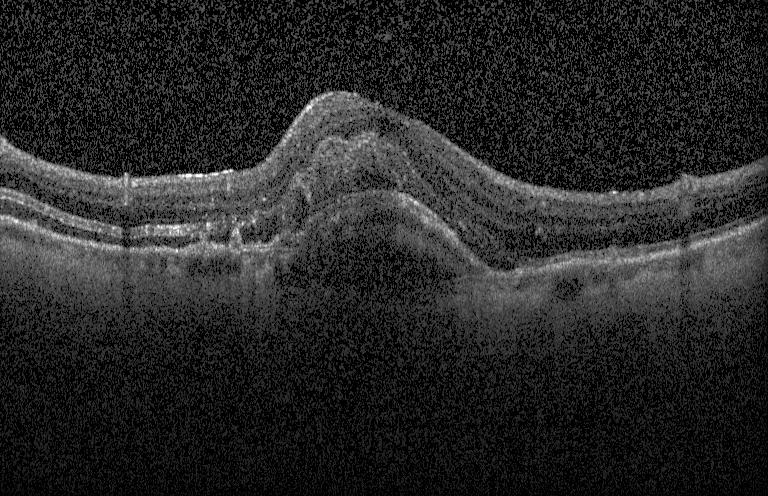
Retinal OCT B-scan. Fovea-centered — The scan shows a choroidal neovascular membrane.